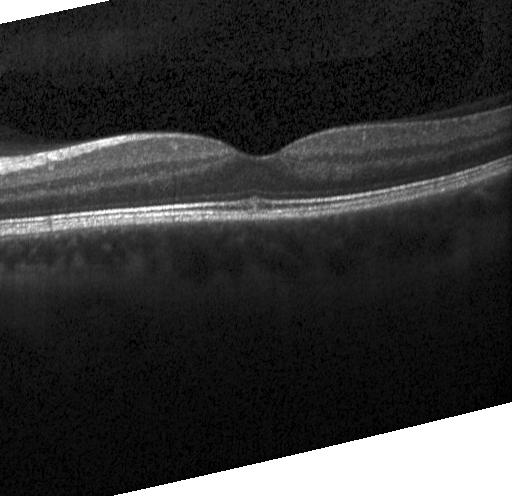

OCT line scan — Impression: no evidence of CNV, DME, or drusen.